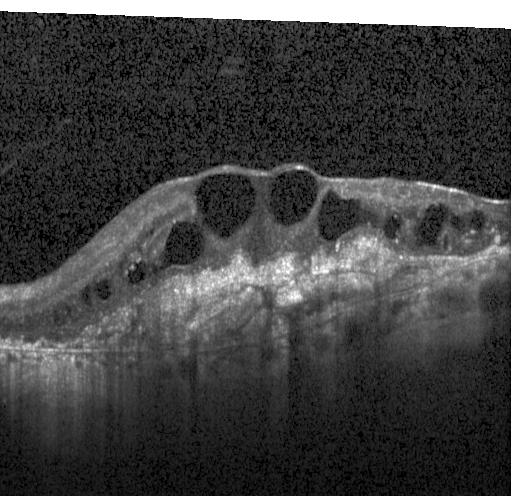

OCT B-scan; Heidelberg Spectralis OCT system; SD-OCT; fovea-centered. Finding: a choroidal neovascular membrane.